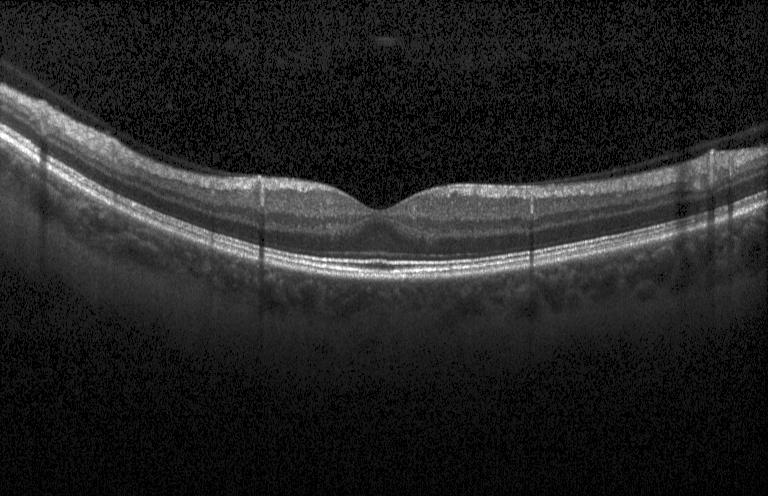 Heidelberg Spectralis OCT system; OCT B-scan.
This B-scan demonstrates no CNV, no DME, and no drusen.